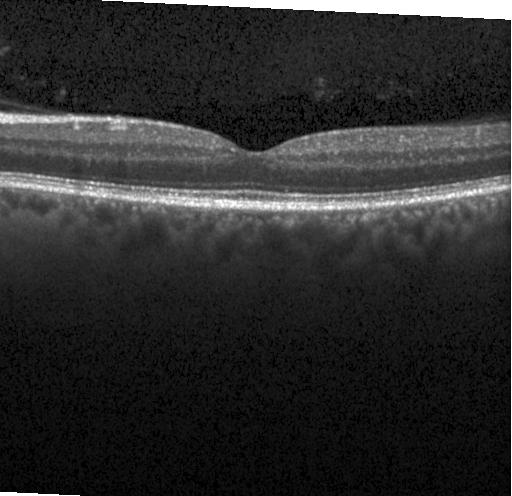

Impression: neither choroidal neovascularization, diabetic macular edema, nor drusen.